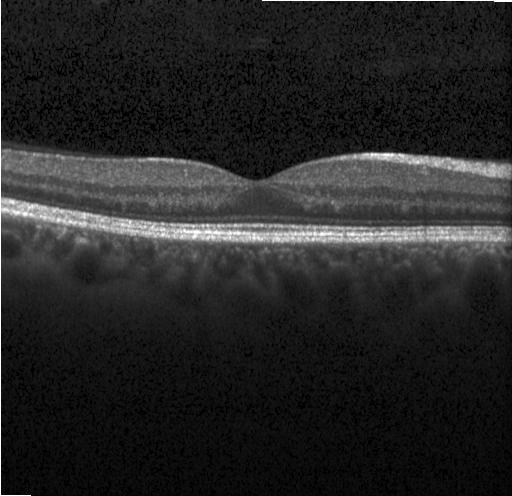
Heidelberg Spectralis. Retinal OCT cross-section. Spectral-domain OCT. This B-scan demonstrates no choroidal neovascularization, no diabetic macular edema, and no drusen.